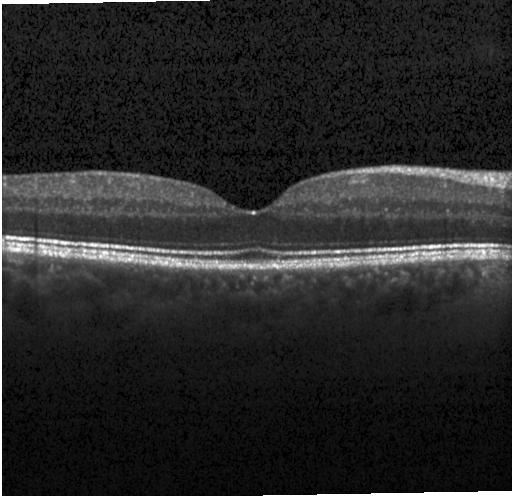 Retinal OCT cross-section · macular scan
Finding: no choroidal neovascularization, no diabetic macular edema, and no drusen.